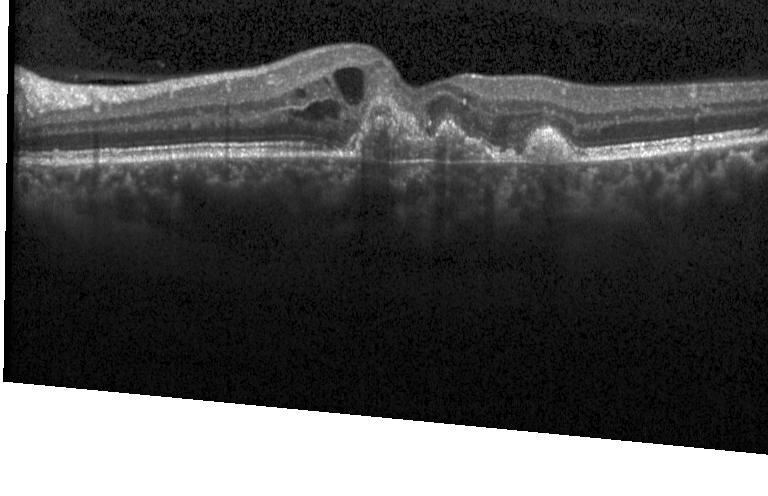

Horizontal scan through the fovea. OCT line scan — Choroidal neovascularization.